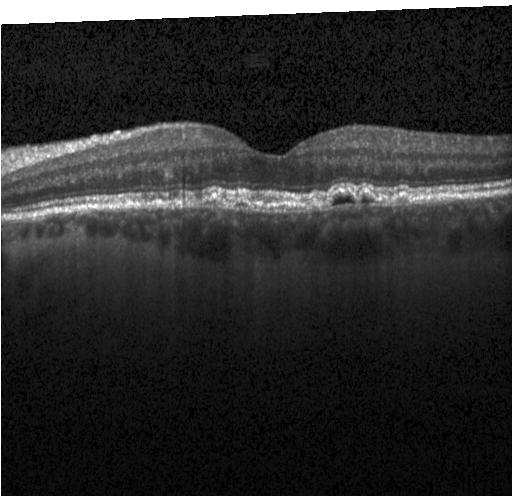 Spectral-domain optical coherence tomography · OCT line scan
Finding: multiple drusen.